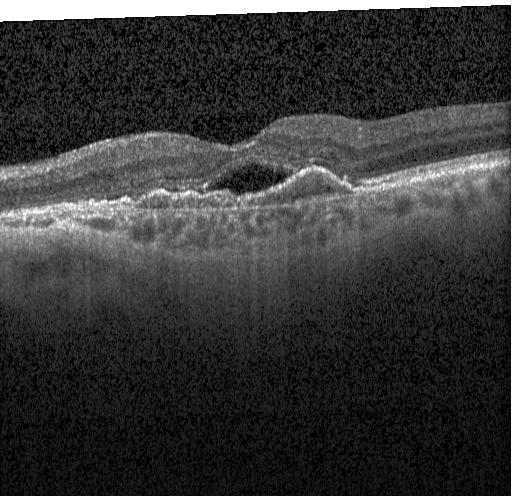 Retinal OCT cross-section, fovea-centered, spectral-domain OCT — Diagnosis: a choroidal neovascular membrane.